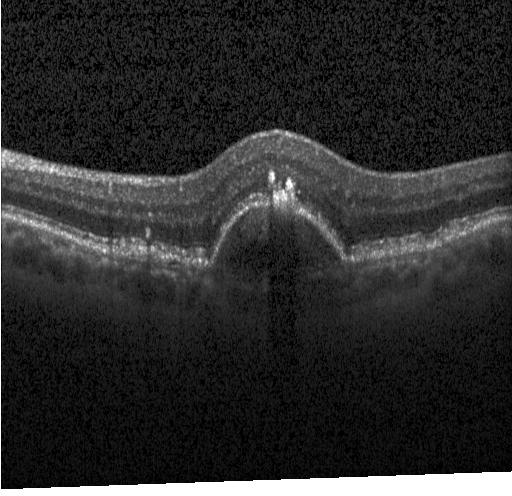
OCT line scan. Macular scan.
Finding: multiple drusen.